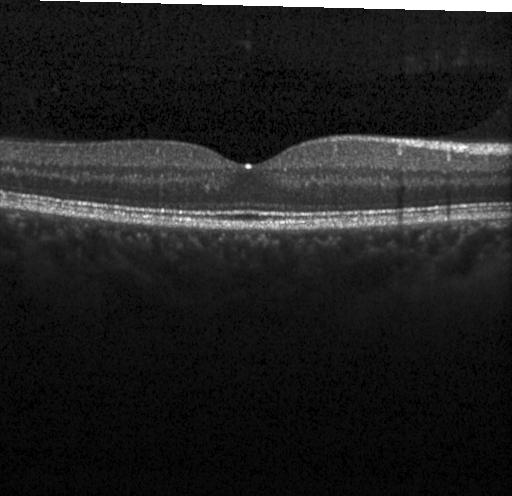

Retinal OCT cross-section
Diagnosis: no CNV, DME, or drusen.